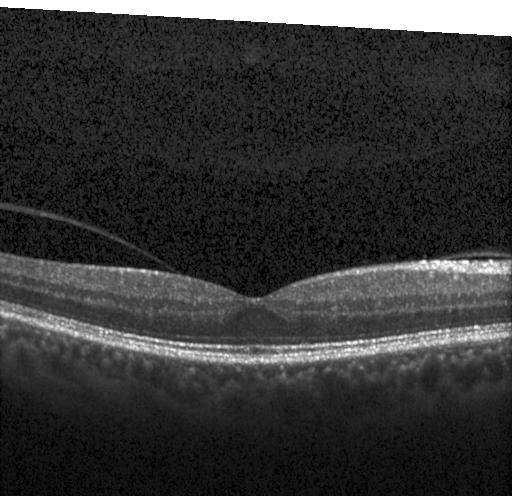
OCT line scan
No CNV, DME, or drusen.